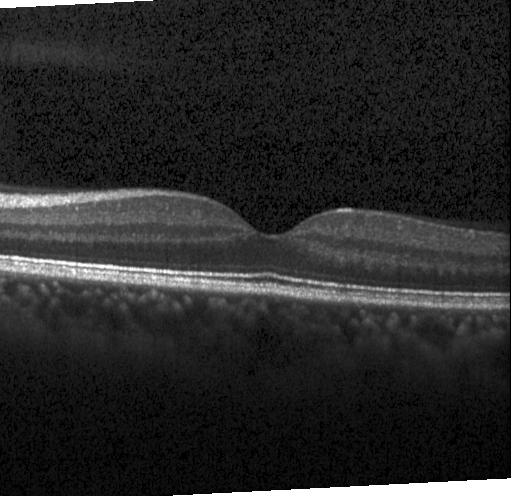
Finding: no choroidal neovascularization, no diabetic macular edema, and no drusen.